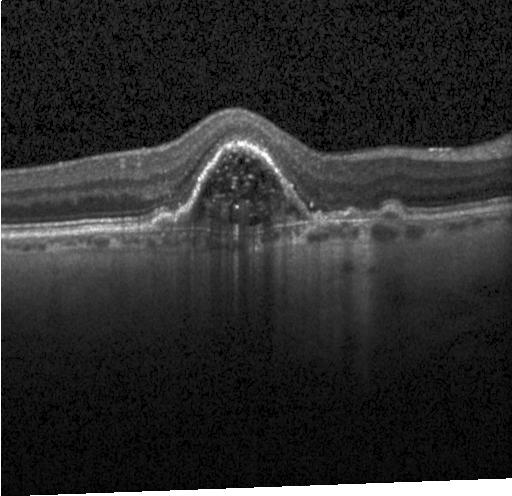
SD-OCT · OCT line scan — Finding: CNV.